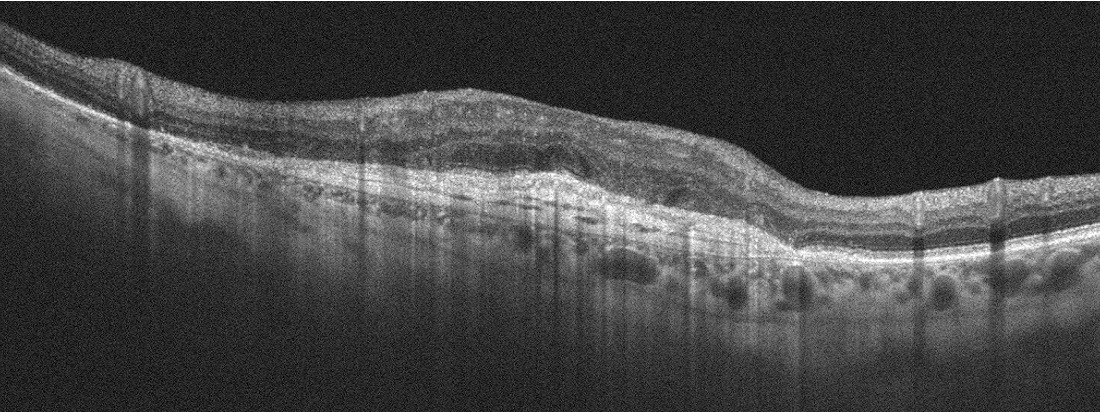
Finding: age-related macular degeneration (AMD).